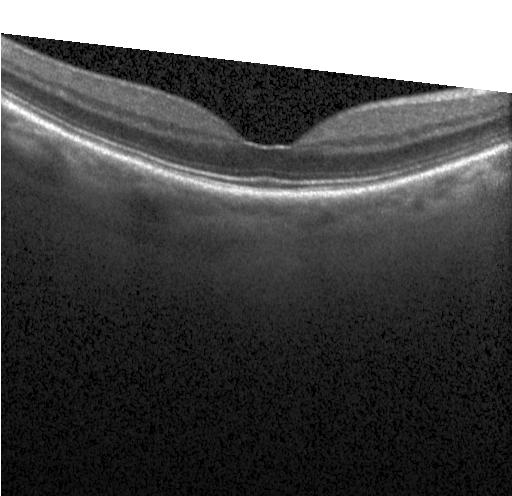

SD-OCT; acquired on a Heidelberg Spectralis; centered on the fovea; retinal OCT B-scan.
Finding: no evidence of CNV, DME, or drusen.